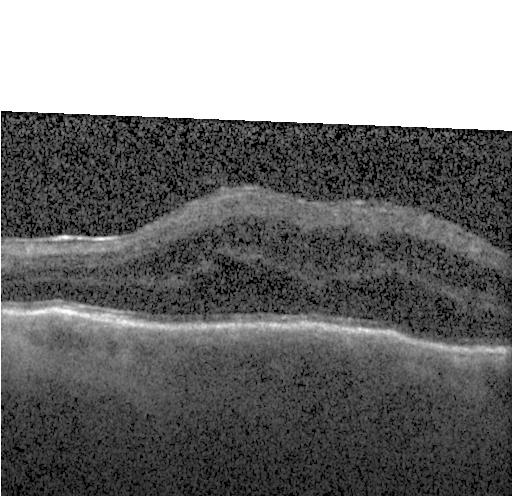 OCT scan showing DME.